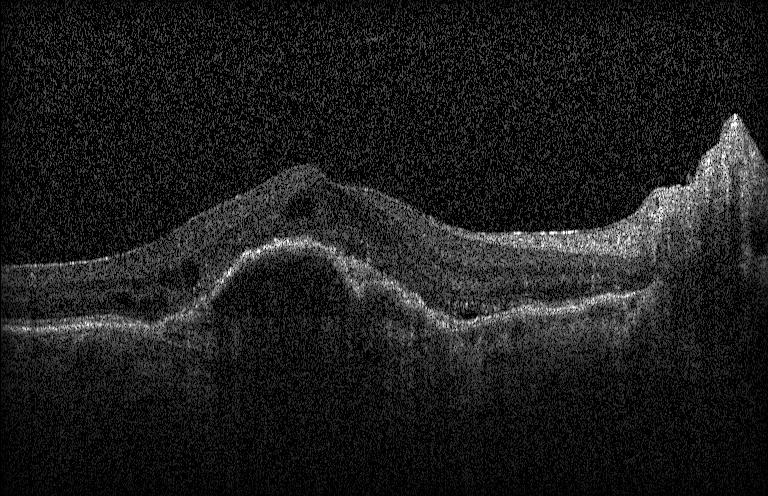 Fovea-centered · instrument: Heidelberg Spectralis · optical coherence tomography scan · spectral-domain optical coherence tomography
OCT finding: a choroidal neovascular membrane.